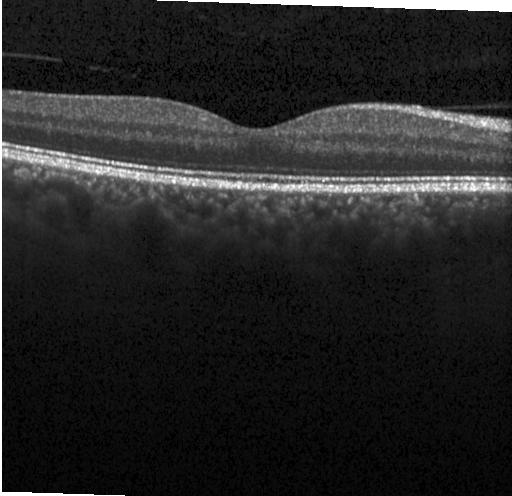
Fovea-centered, optical coherence tomography B-scan — Impression: no evidence of CNV, DME, or drusen.